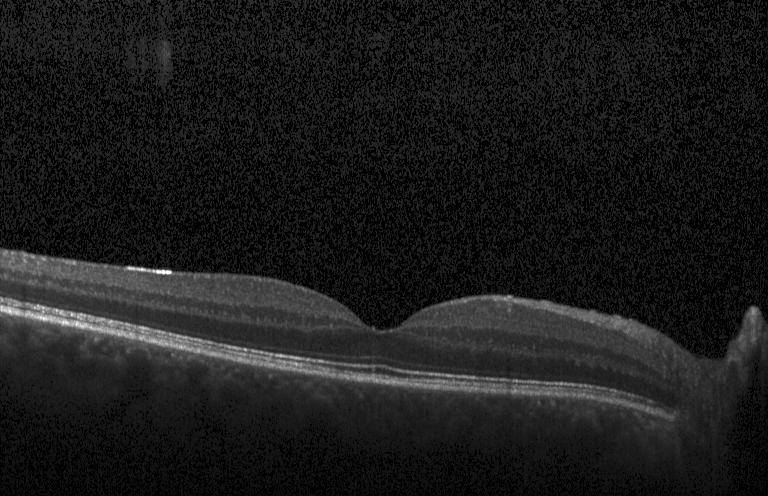
Fovea-centered. Optical coherence tomography scan. Spectral-domain optical coherence tomography. Acquired on a Heidelberg Spectralis.
OCT finding: no evidence of choroidal neovascularization, diabetic macular edema, or drusen.